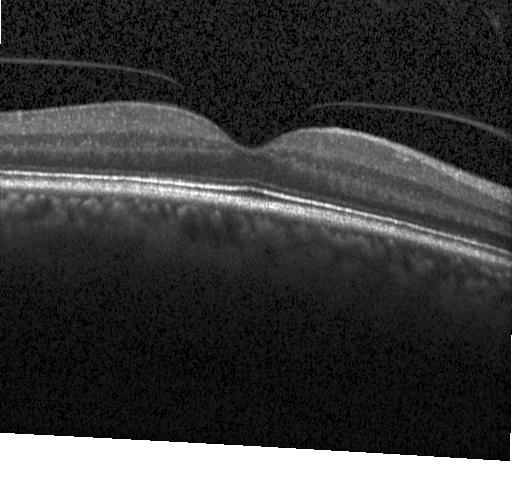
Retinal OCT cross-section. The scan shows no choroidal neovascularization, no diabetic macular edema, and no drusen.